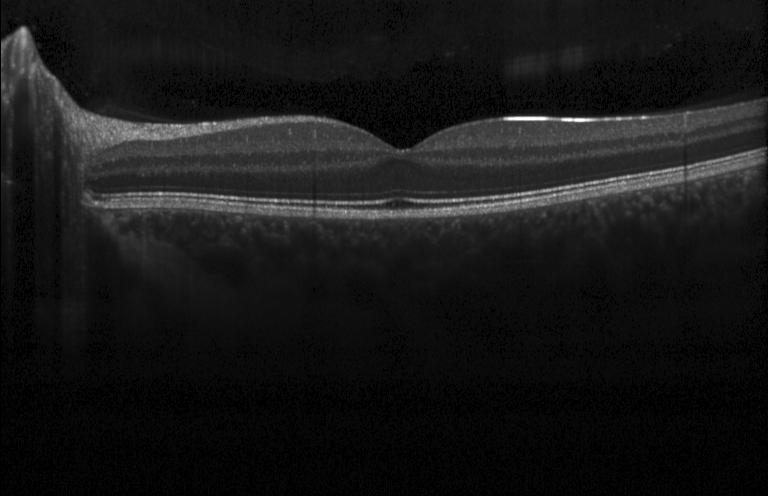

Macular scan; spectral-domain OCT; Heidelberg Spectralis OCT system; optical coherence tomography B-scan. Finding: no choroidal neovascularization, no diabetic macular edema, and no drusen.